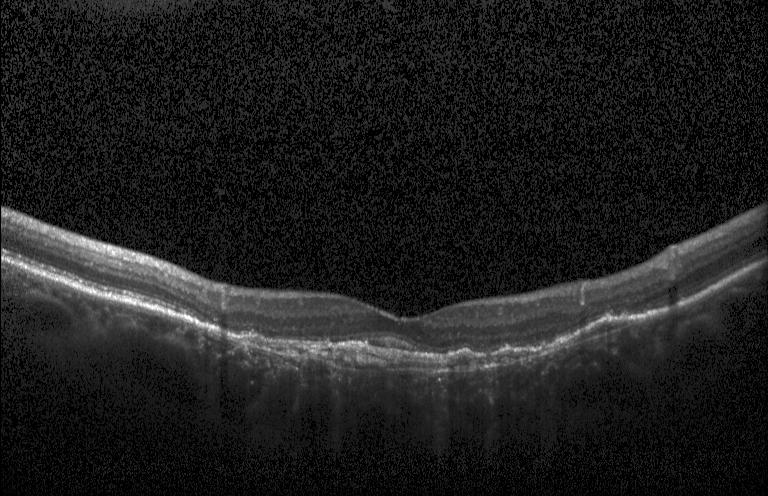

Impression: CNV.